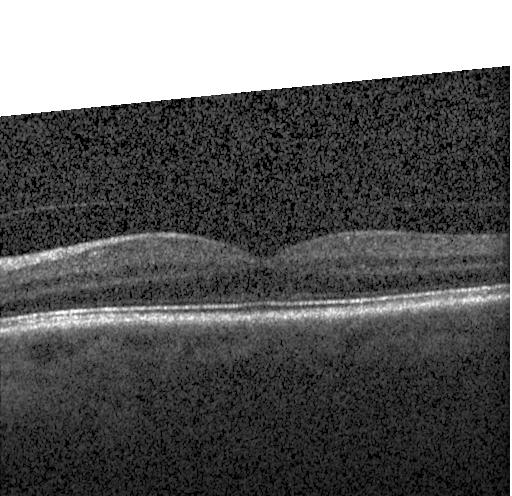 SD-OCT, OCT B-scan, Heidelberg Spectralis
The scan shows no evidence of CNV, DME, or drusen.